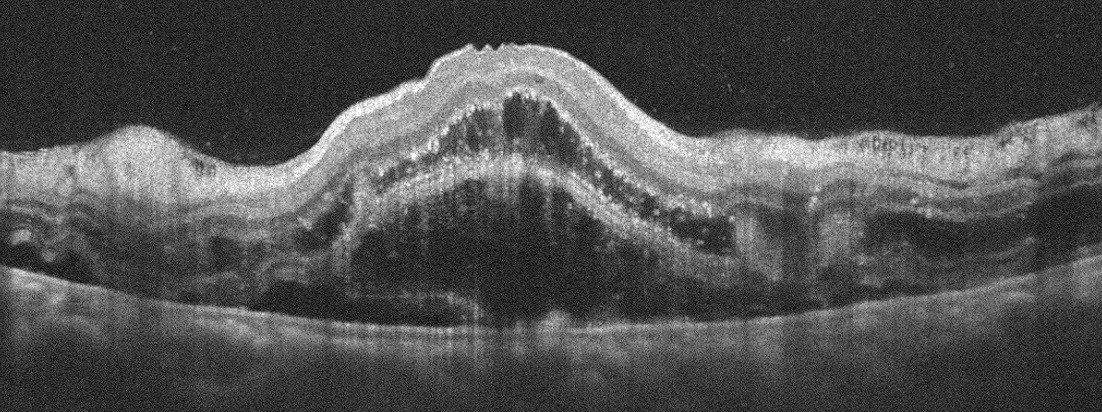 OCT scan showing retinal vein occlusion (RVO).